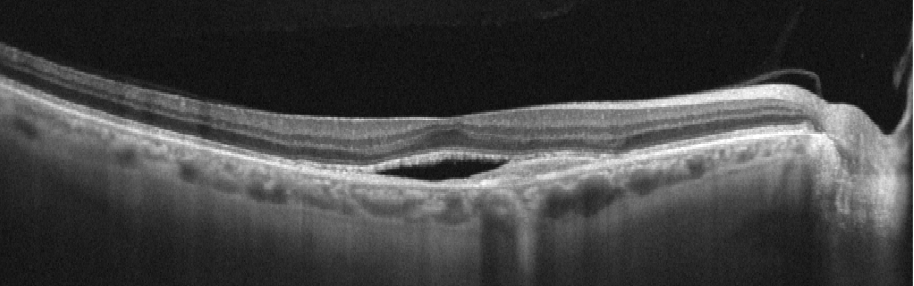 This B-scan demonstrates age-related macular degeneration.